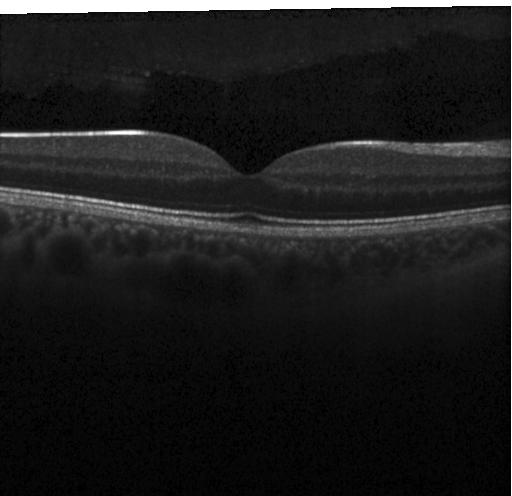

This B-scan demonstrates no choroidal neovascularization, diabetic macular edema, or drusen.